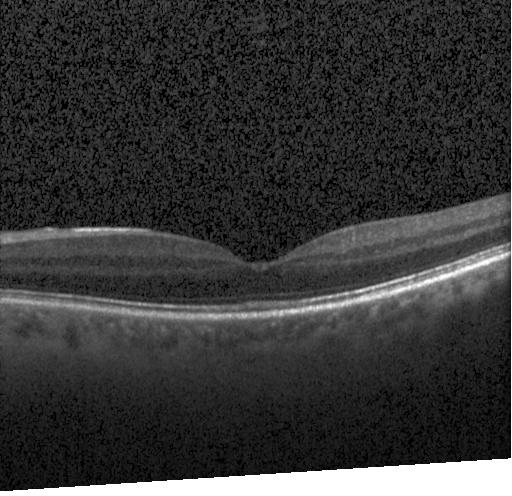
Diagnosis: no evidence of choroidal neovascularization, diabetic macular edema, or drusen.